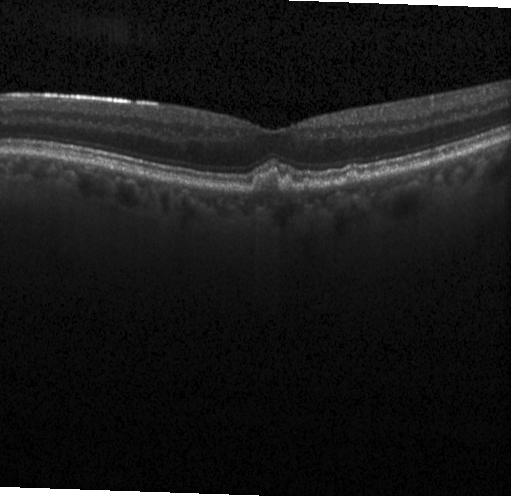 Spectral-domain OCT B-scan: multiple drusen.